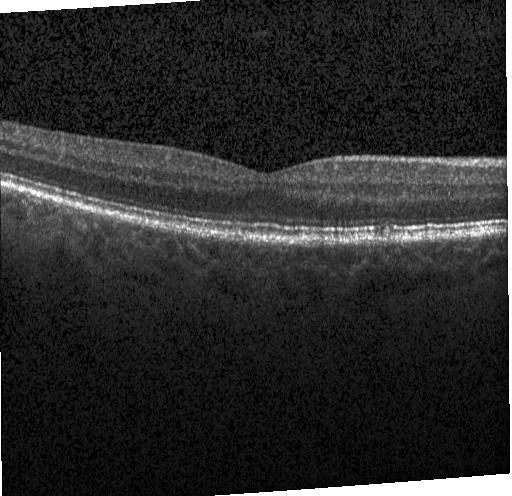

Macular OCT: drusen.